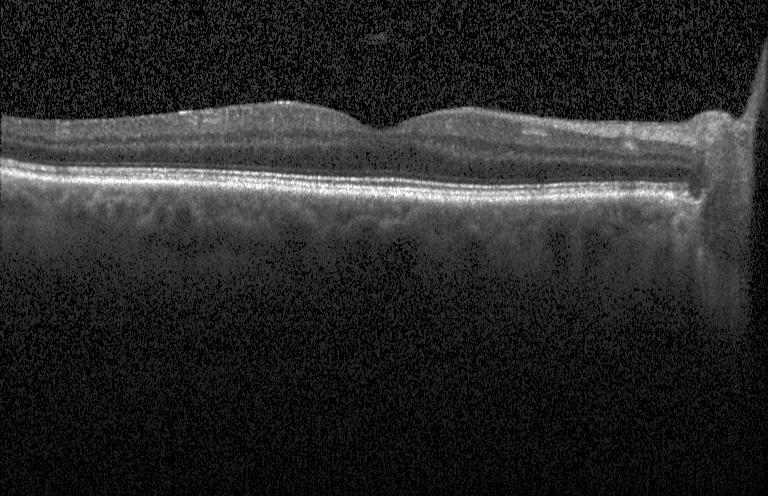

Macular OCT: no choroidal neovascularization, diabetic macular edema, or drusen.